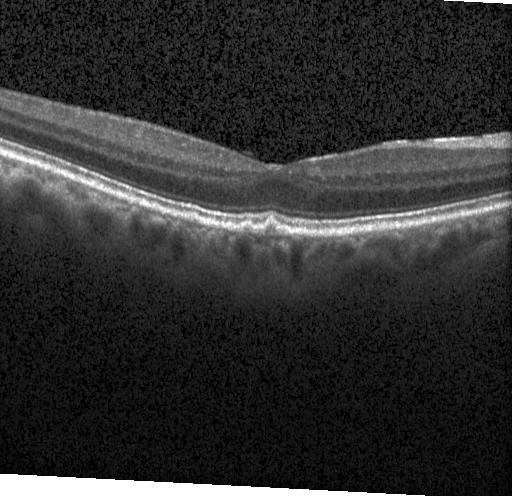
The scan shows multiple drusen.